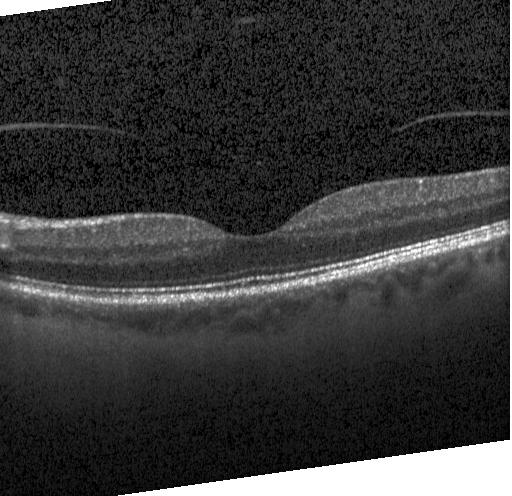 Diagnosis: neither choroidal neovascularization, diabetic macular edema, nor drusen.